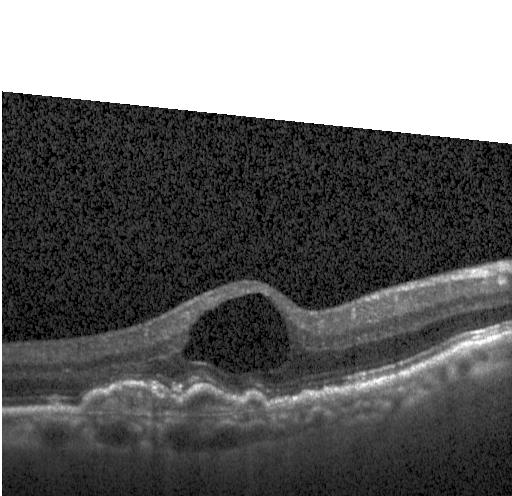
Retinal OCT cross-section
A choroidal neovascular membrane.